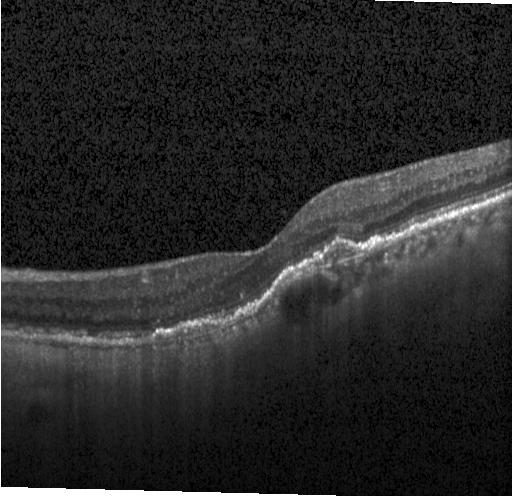 Optical coherence tomography B-scan. Diagnosis: choroidal neovascularization (CNV).